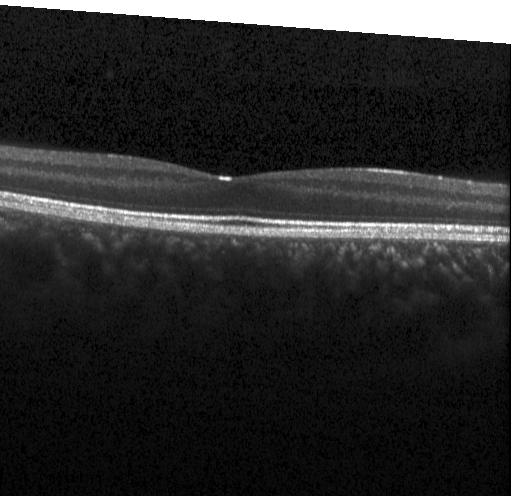 Finding: no CNV, no DME, and no drusen.